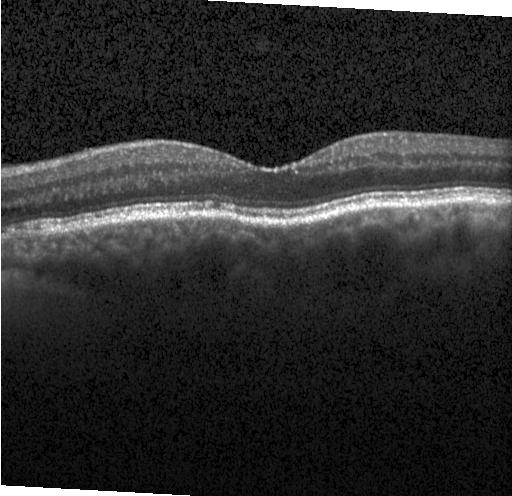
Acquired on a Heidelberg Spectralis. OCT line scan. Spectral-domain optical coherence tomography
Assessment: no choroidal neovascularization, diabetic macular edema, or drusen.